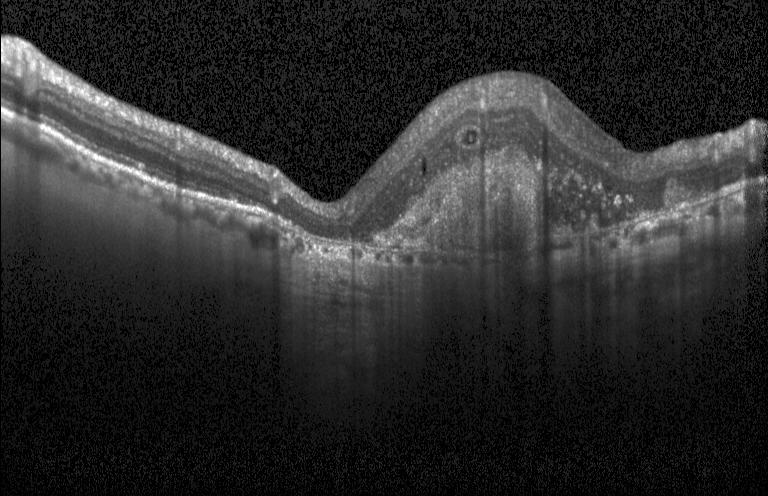 OCT finding: a choroidal neovascular membrane.